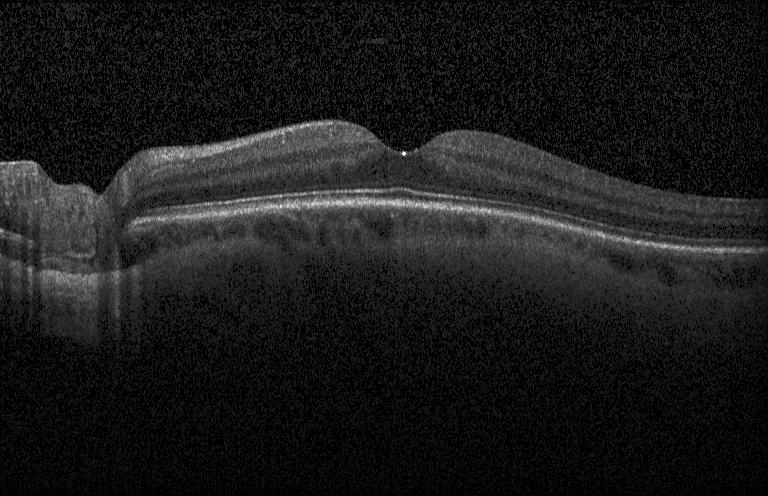
OCT B-scan — Finding: no choroidal neovascularization, no diabetic macular edema, and no drusen.